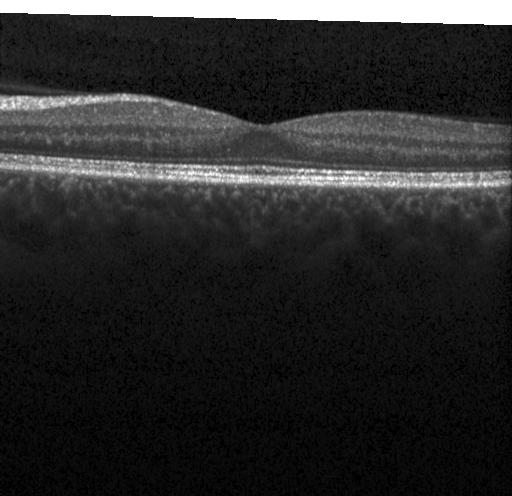

Optical coherence tomography scan; horizontal scan through the fovea.
Diagnosis: neither choroidal neovascularization, diabetic macular edema, nor drusen.